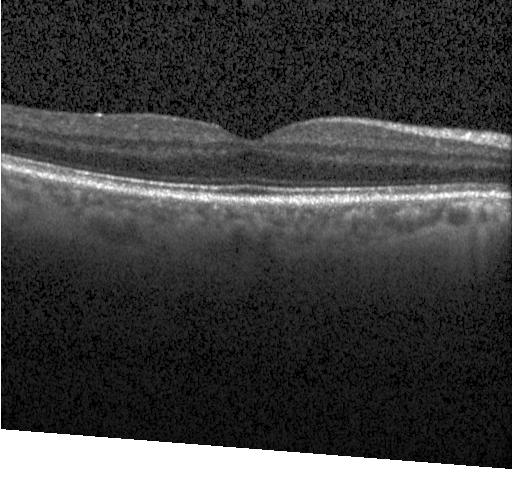

Retinal OCT B-scan; Heidelberg Spectralis OCT system; SD-OCT. This B-scan demonstrates no CNV, DME, or drusen.